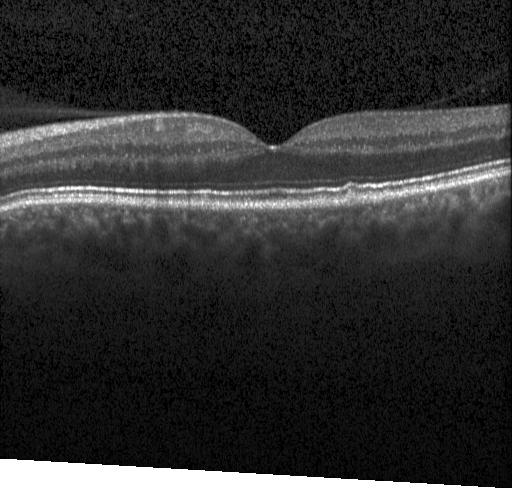

Macular OCT demonstrating drusen.